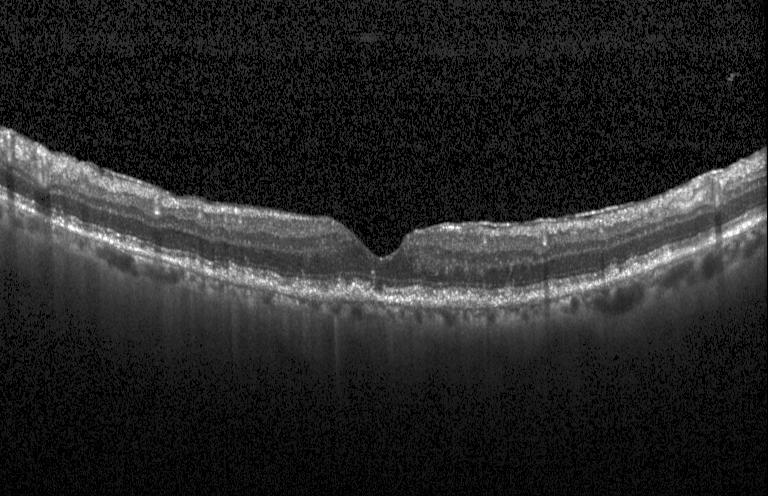
Impression: drusen.